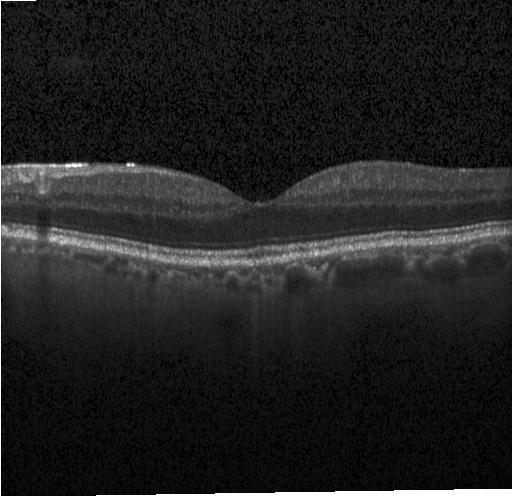 Heidelberg Spectralis OCT system; SD-OCT; optical coherence tomography B-scan; through the macula
Impression: neither choroidal neovascularization, diabetic macular edema, nor drusen.